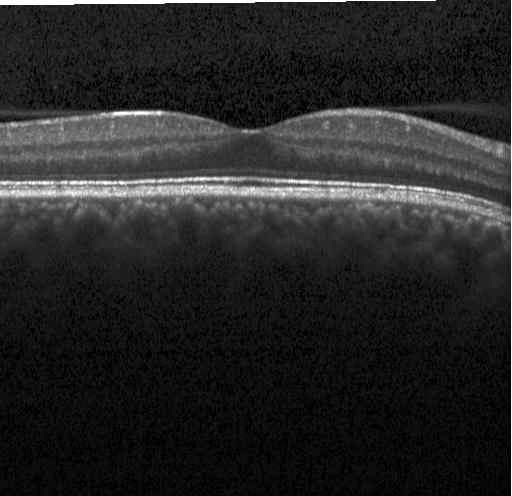 OCT scan showing no evidence of choroidal neovascularization, diabetic macular edema, or drusen.